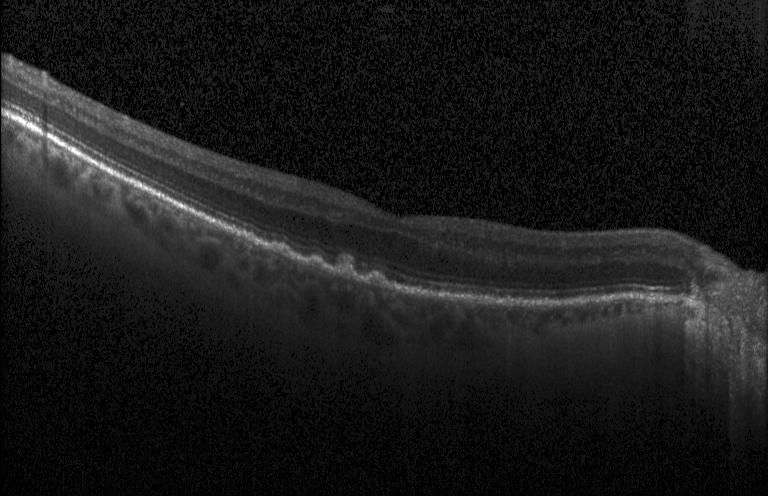

Impression: sub-RPE drusenoid deposits.